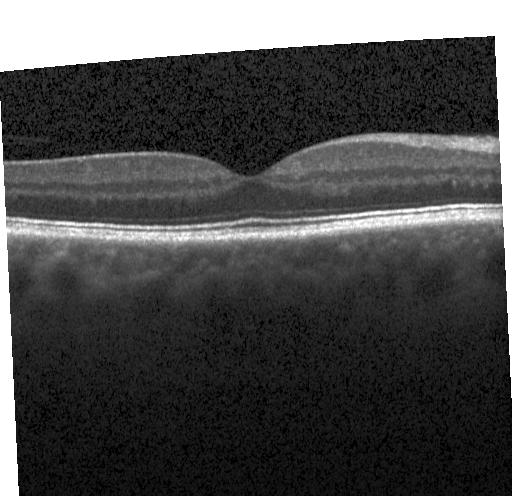
Macular OCT demonstrating no evidence of choroidal neovascularization, diabetic macular edema, or drusen.